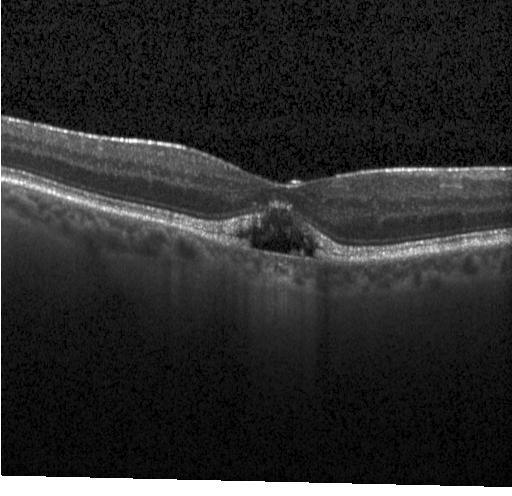 Assessment: choroidal neovascularization.